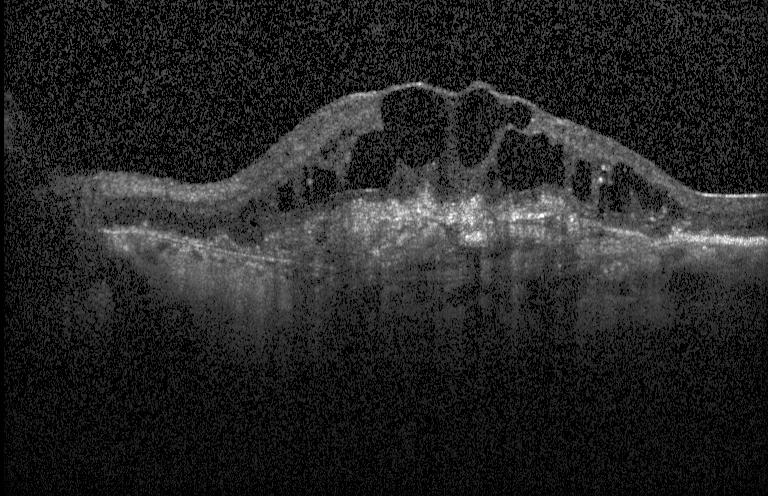
Retinal OCT cross-section showing choroidal neovascularization (CNV).